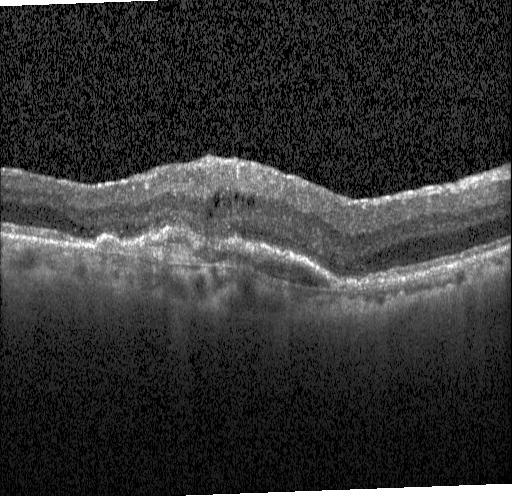
Dx: choroidal neovascularization (CNV).